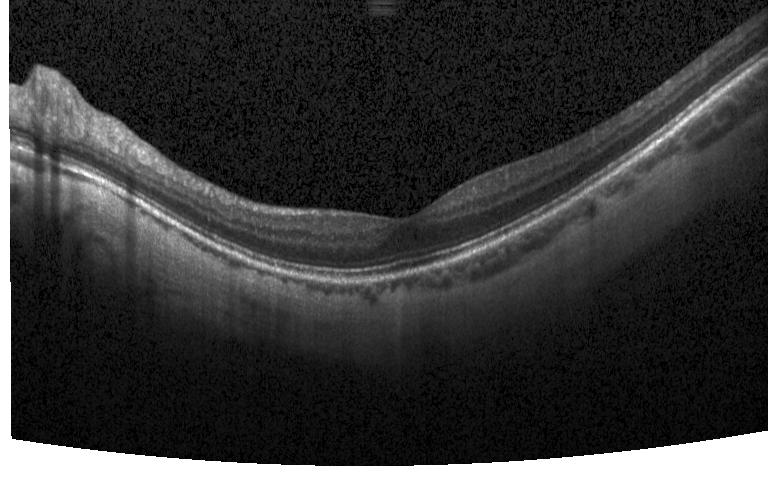

Instrument: Heidelberg Spectralis. Retinal OCT cross-section. Assessment: no evidence of choroidal neovascularization, diabetic macular edema, or drusen.